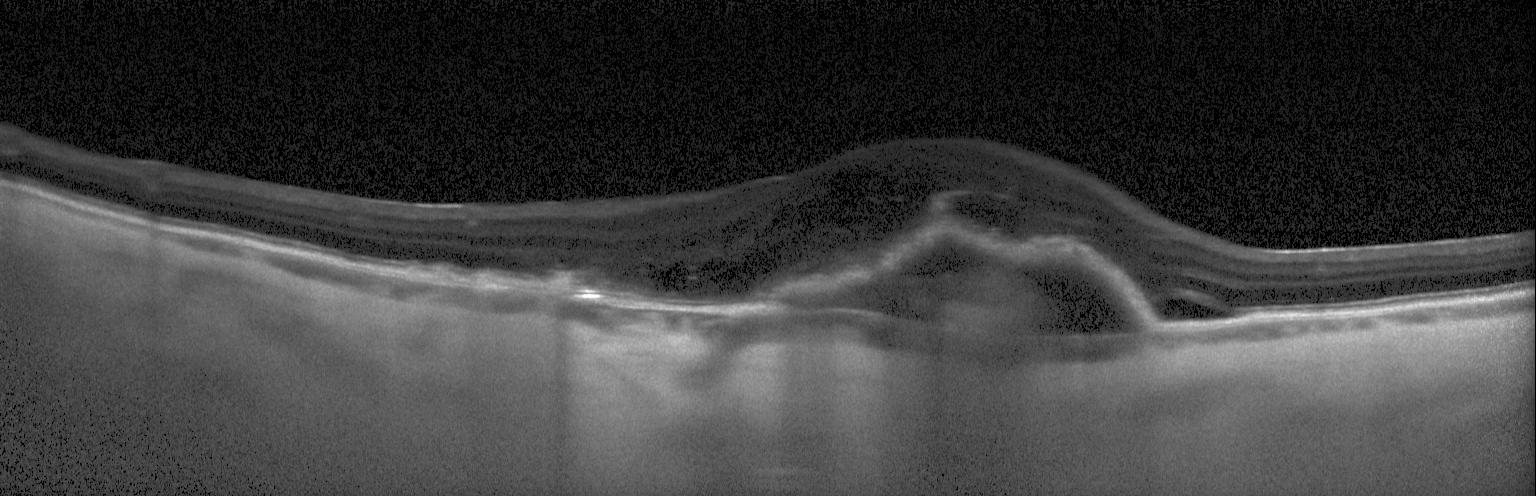

Fovea-centered · retinal OCT cross-section · spectral-domain OCT — Diagnosis: choroidal neovascularization.